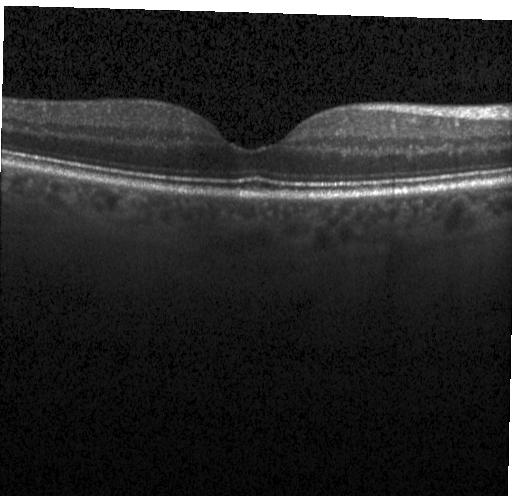
Spectral-domain OCT; acquired on a Heidelberg Spectralis; OCT line scan.
Diagnosis: no choroidal neovascularization, no diabetic macular edema, and no drusen.